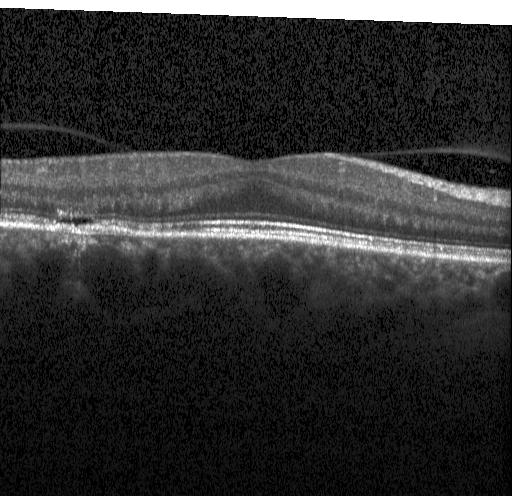

Heidelberg Spectralis OCT system; retinal OCT cross-section.
Impression: a choroidal neovascular membrane.